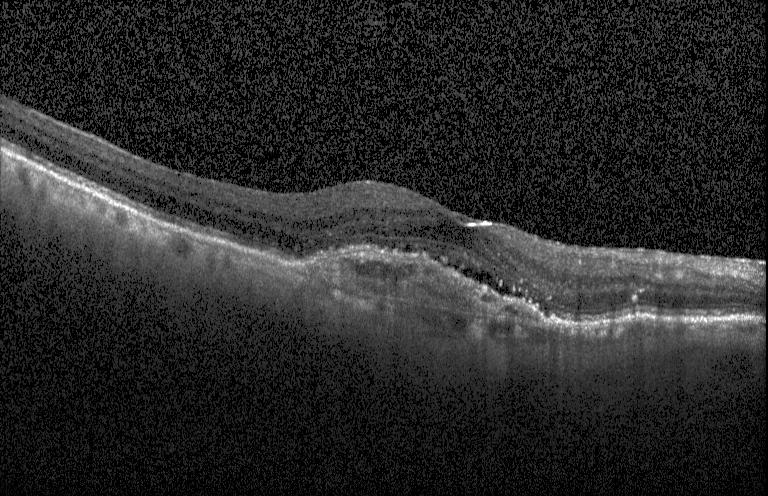 Retinal OCT cross-section; spectral-domain OCT — This B-scan demonstrates a choroidal neovascular membrane.